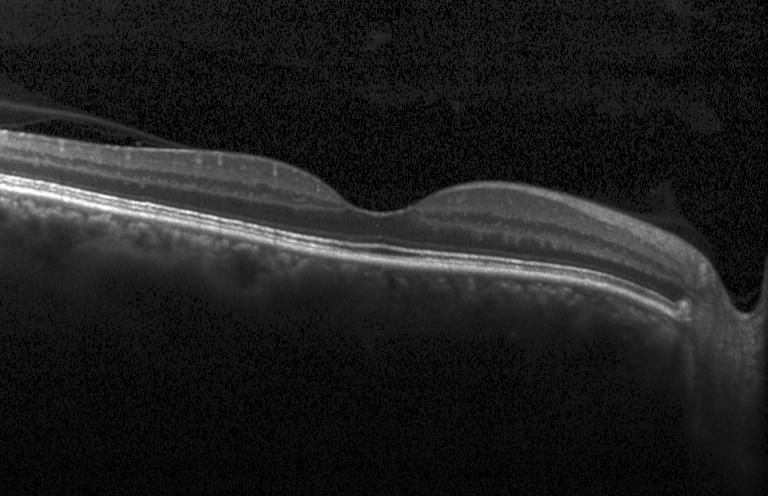
OCT B-scan, spectral-domain OCT, instrument: Heidelberg Spectralis
Assessment: no choroidal neovascularization, diabetic macular edema, or drusen.